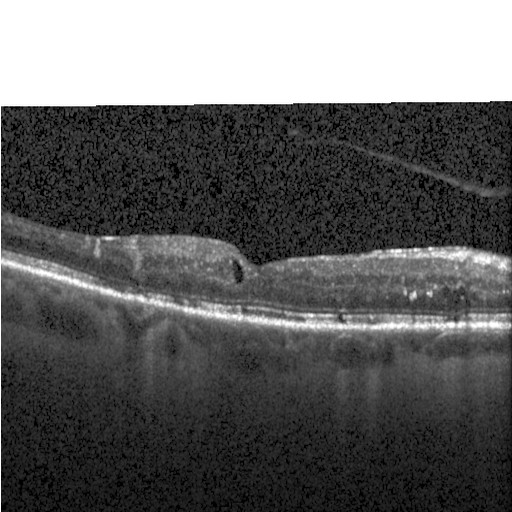
Finding: diabetic macular edema.